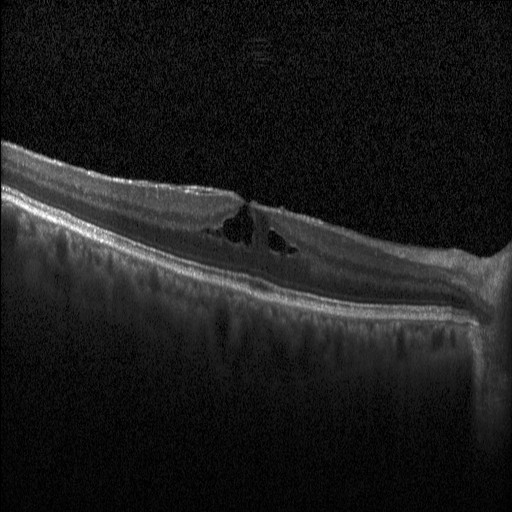 OCT line scan, SD-OCT — Assessment: diabetic macular edema (DME).